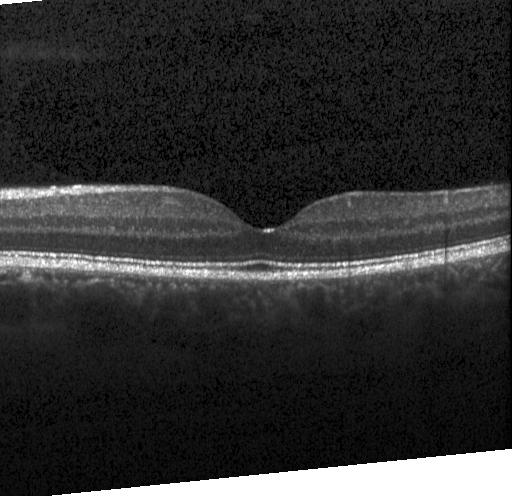 Fovea-centered. Spectral-domain OCT. Optical coherence tomography scan — Finding: no choroidal neovascularization, diabetic macular edema, or drusen.